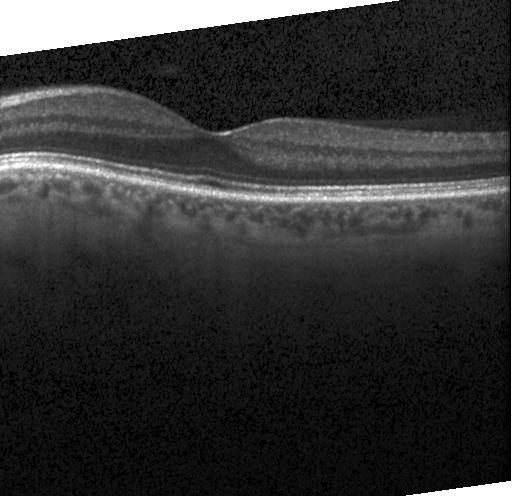
Spectral-domain optical coherence tomography; OCT line scan — Diagnosis: no CNV, DME, or drusen.